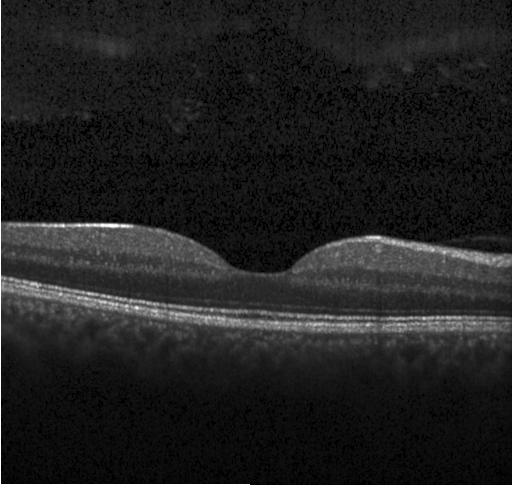
Optical coherence tomography scan
Finding: no evidence of choroidal neovascularization, diabetic macular edema, or drusen.